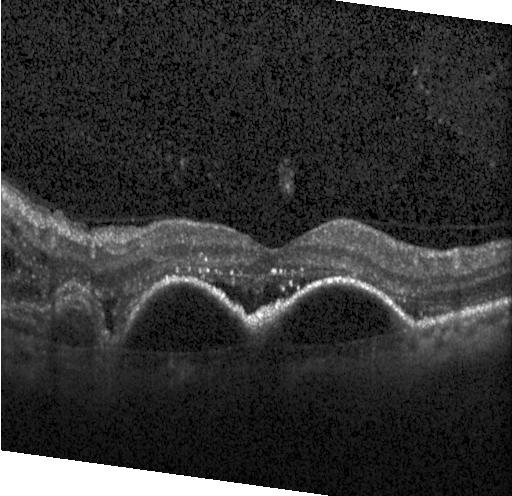
OCT B-scan.
Finding: choroidal neovascularization (CNV).